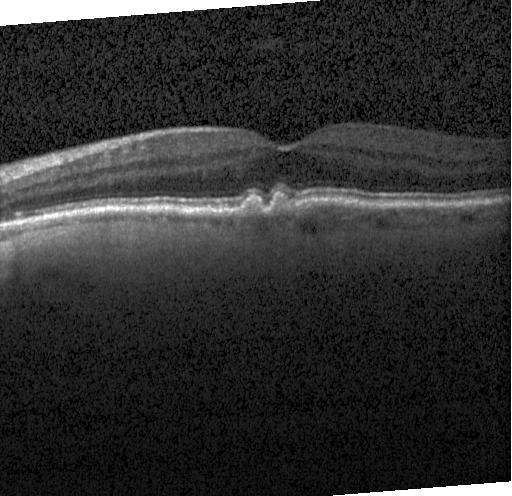
Impression: drusen.